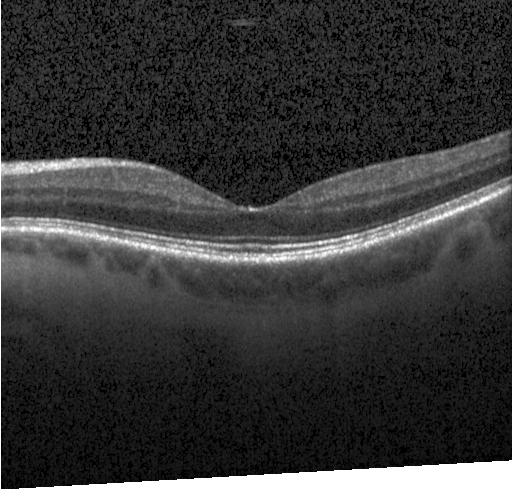

Assessment: no CNV, no DME, and no drusen.